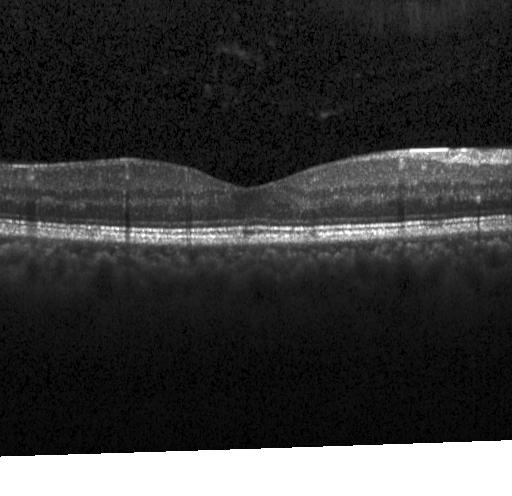

Impression: no evidence of choroidal neovascularization, diabetic macular edema, or drusen.